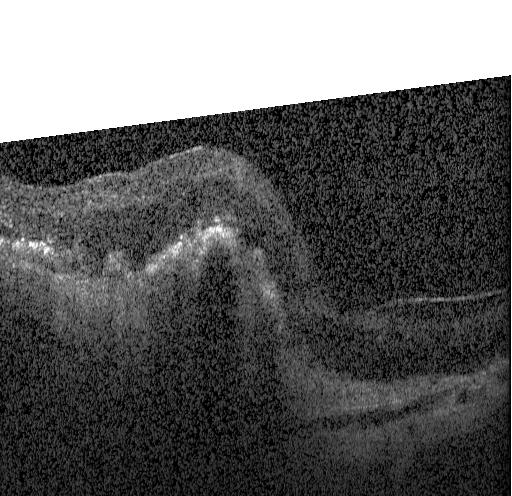 Centered on the fovea · OCT B-scan — Macular OCT: a choroidal neovascular membrane.